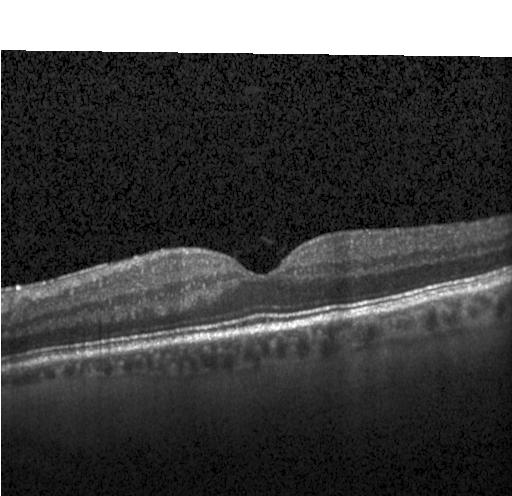
Macular OCT demonstrating no choroidal neovascularization, diabetic macular edema, or drusen.